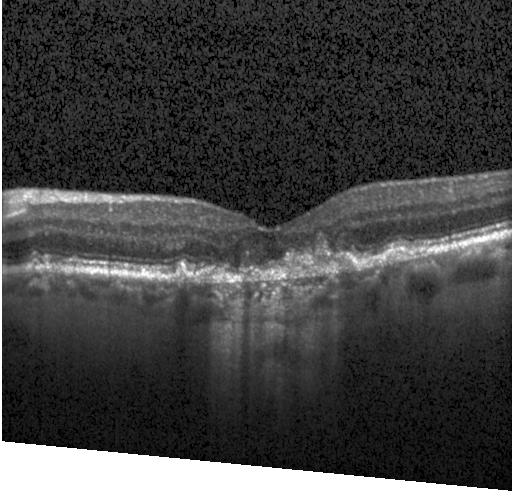
Assessment: choroidal neovascularization.